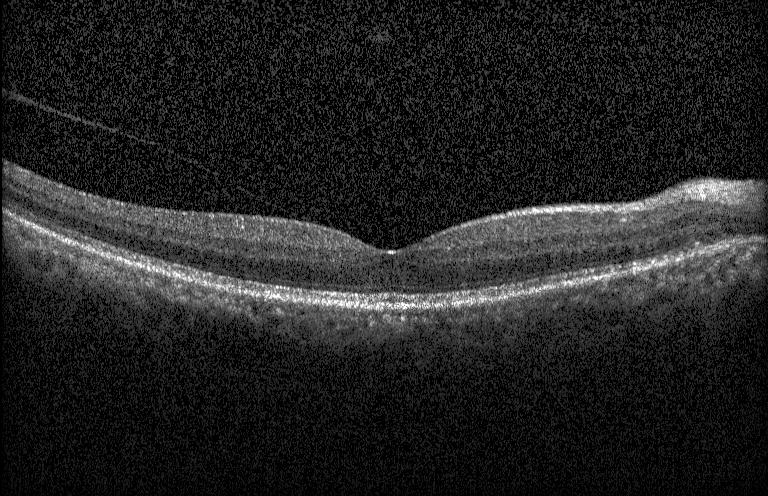

Optical coherence tomography B-scan. No choroidal neovascularization, diabetic macular edema, or drusen.